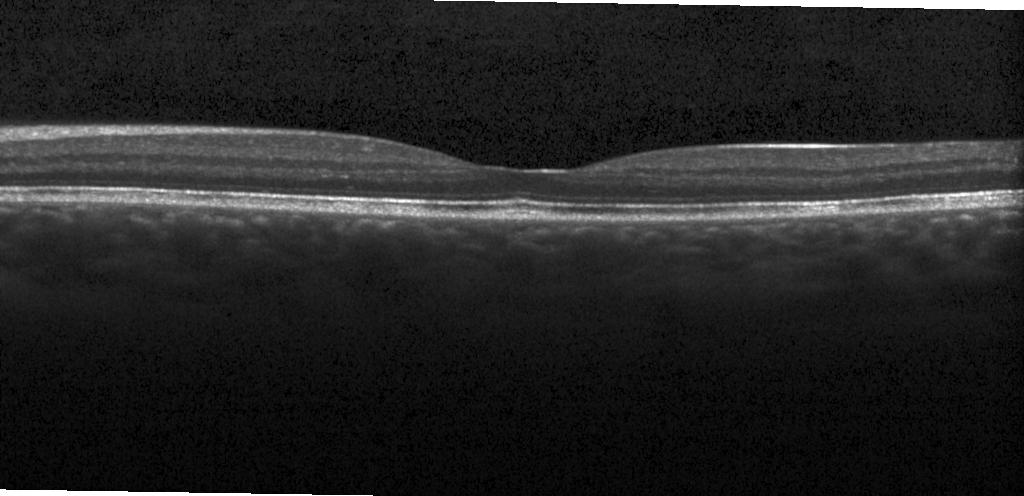

Spectral-domain optical coherence tomography · acquired on a Heidelberg Spectralis · OCT B-scan · through the macula — Impression: neither CNV, DME, nor drusen.